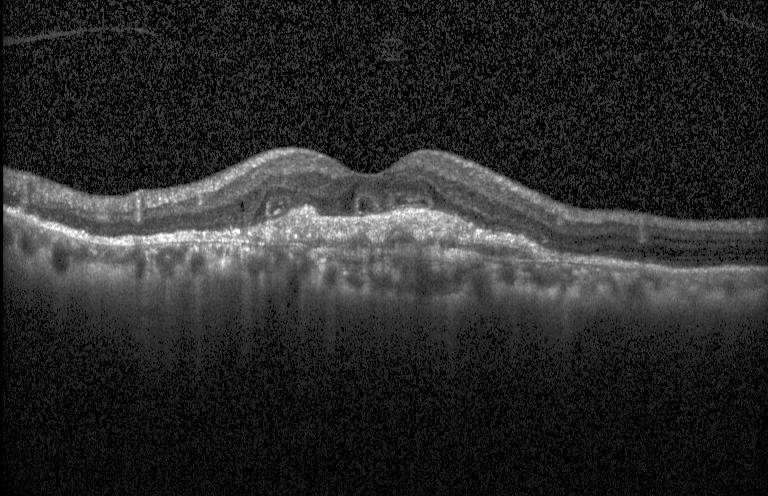 Retinal OCT cross-section. Fovea-centered. Spectral-domain optical coherence tomography. Heidelberg Spectralis OCT system — Dx: choroidal neovascularization.